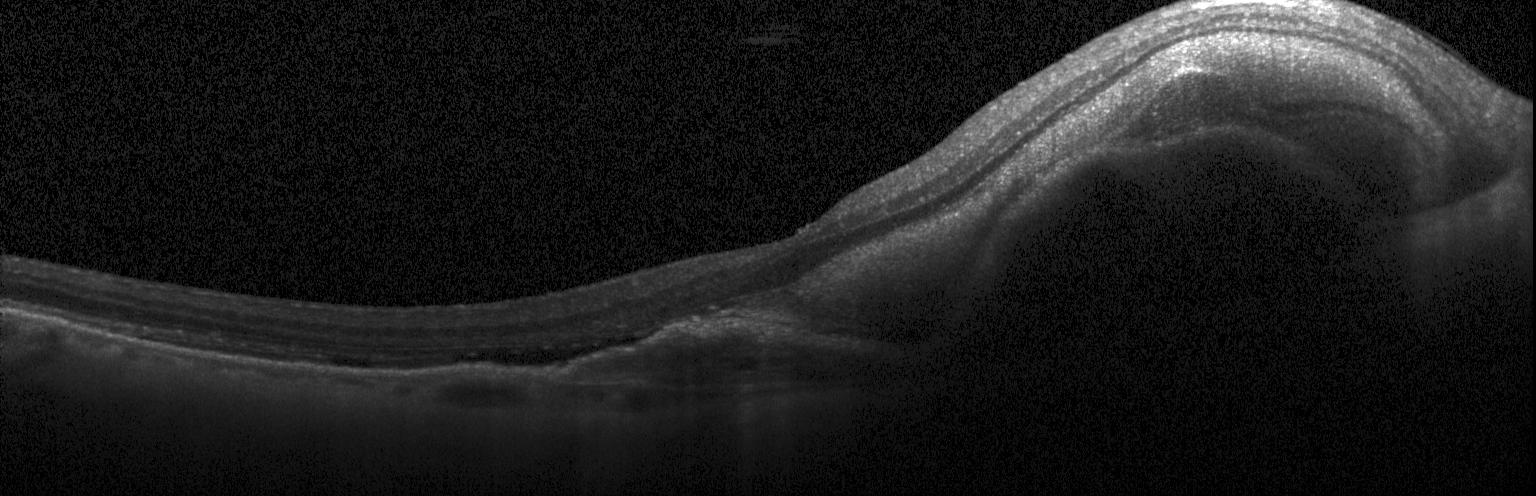 Centered on the fovea; SD-OCT; optical coherence tomography B-scan.
Assessment: choroidal neovascularization (CNV).